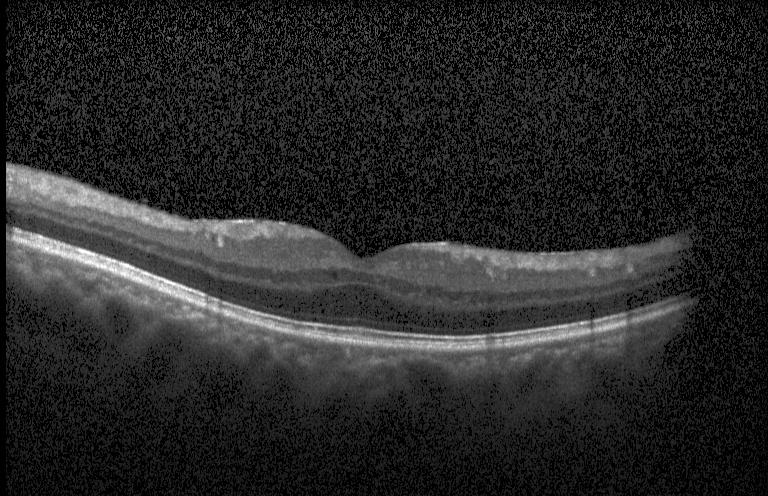

Impression: no choroidal neovascularization, no diabetic macular edema, and no drusen.